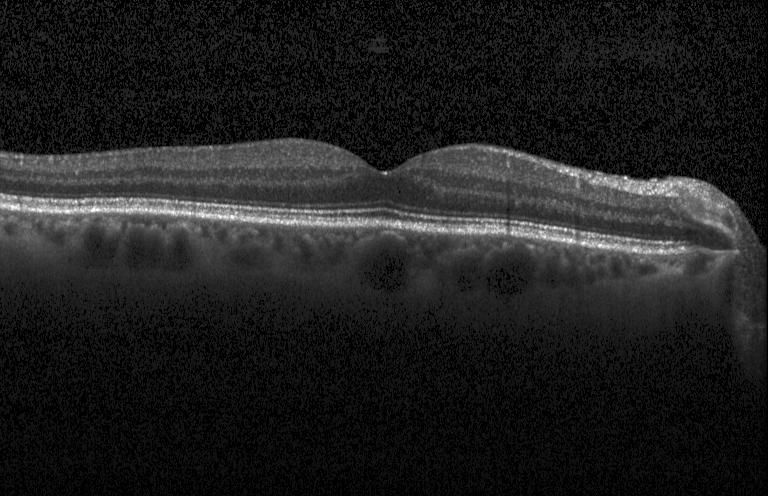 Retinal OCT B-scan. SD-OCT
Impression: no choroidal neovascularization, no diabetic macular edema, and no drusen.